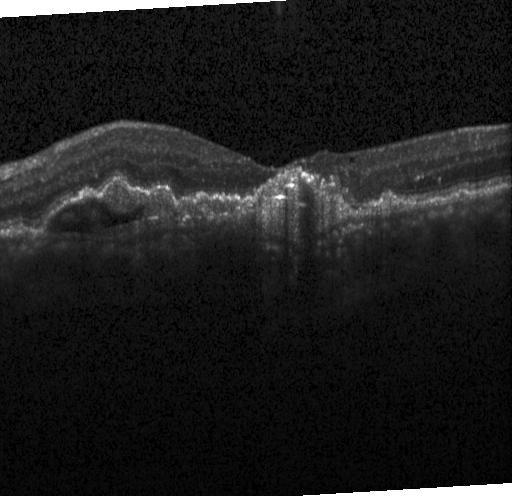

Impression: a choroidal neovascular membrane.